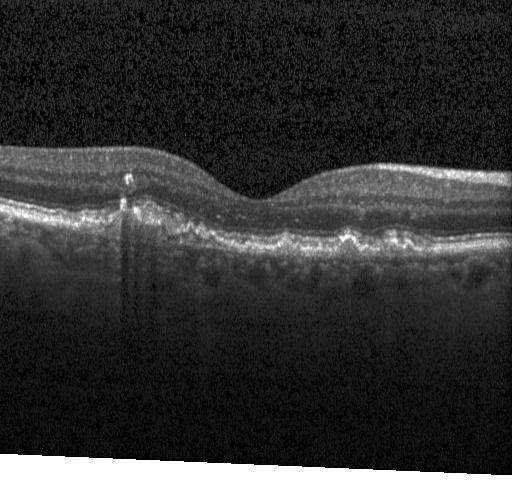
OCT B-scan showing choroidal neovascularization (CNV).